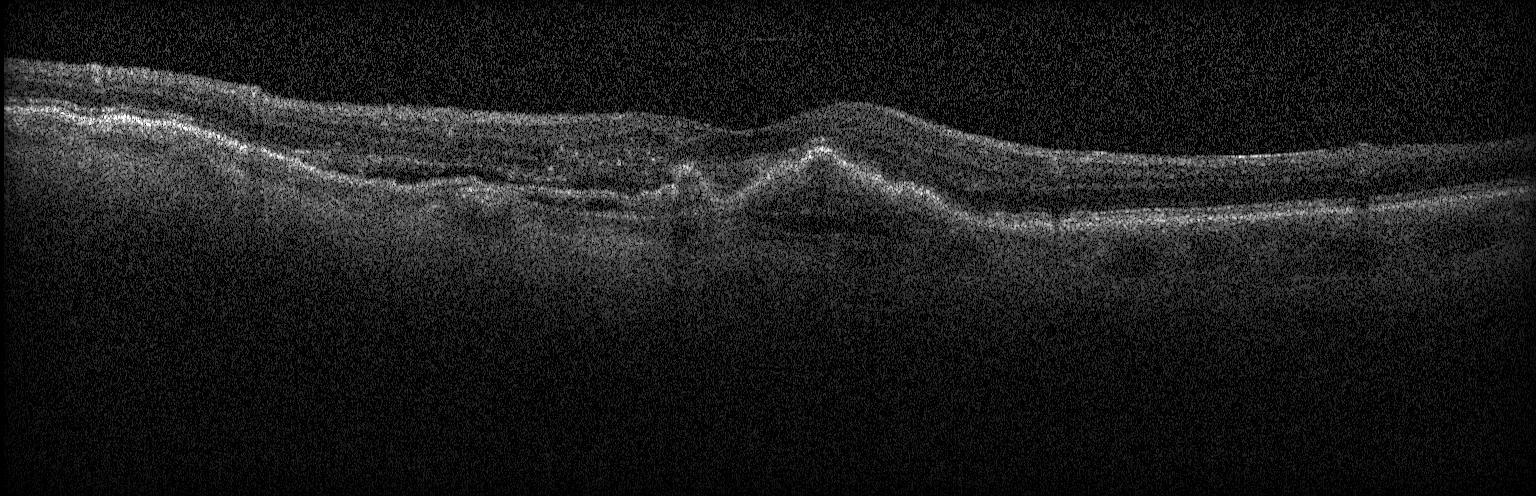 Optical coherence tomography B-scan
Macular OCT: a choroidal neovascular membrane.